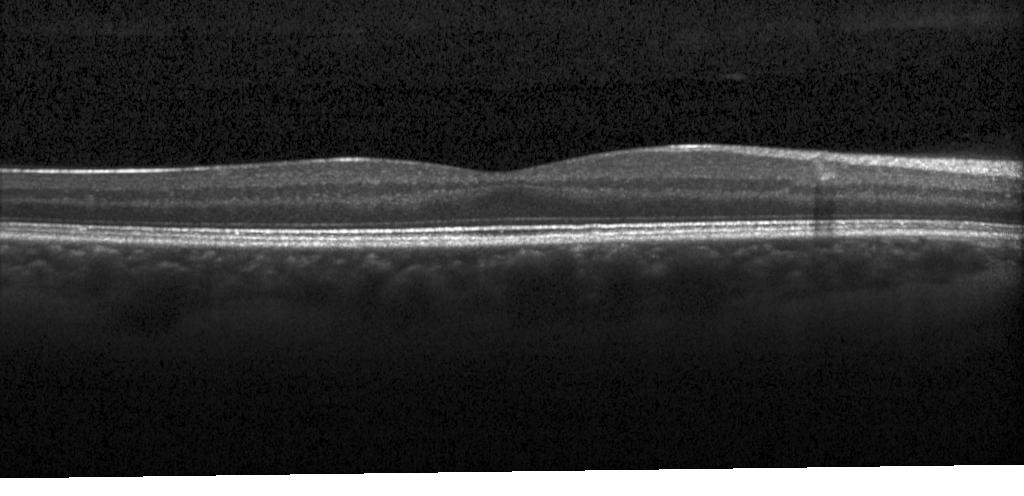

OCT finding: no choroidal neovascularization, diabetic macular edema, or drusen.